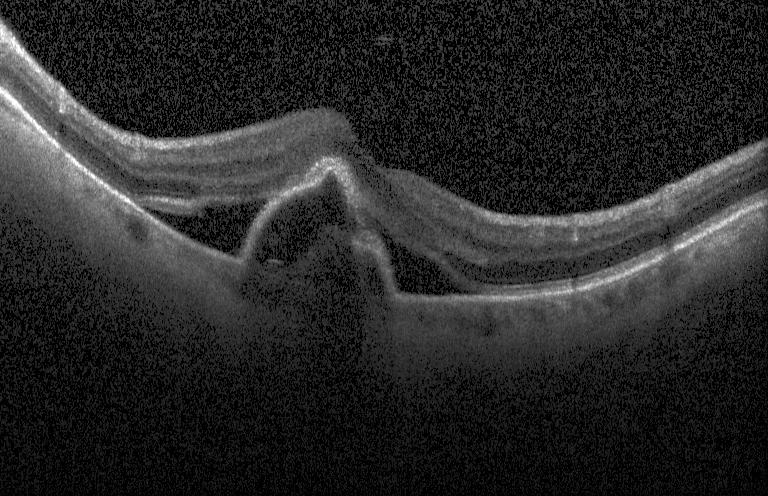 Fovea-centered · optical coherence tomography scan · instrument: Heidelberg Spectralis. Finding: a choroidal neovascular membrane.